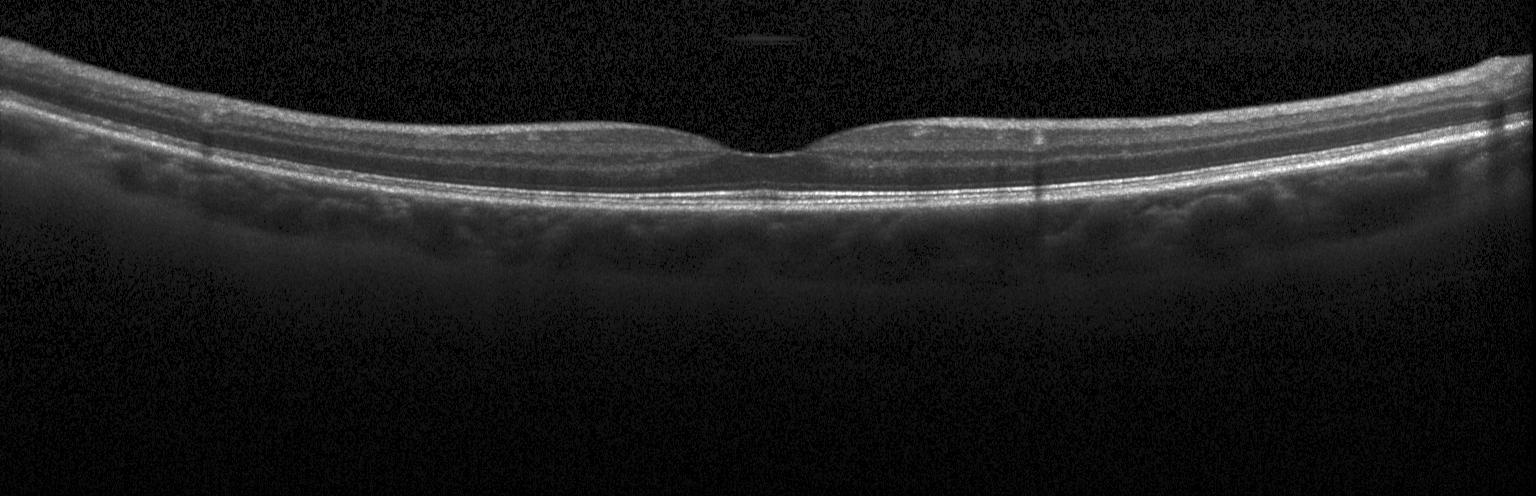 OCT B-scan. OCT finding: no evidence of choroidal neovascularization, diabetic macular edema, or drusen.